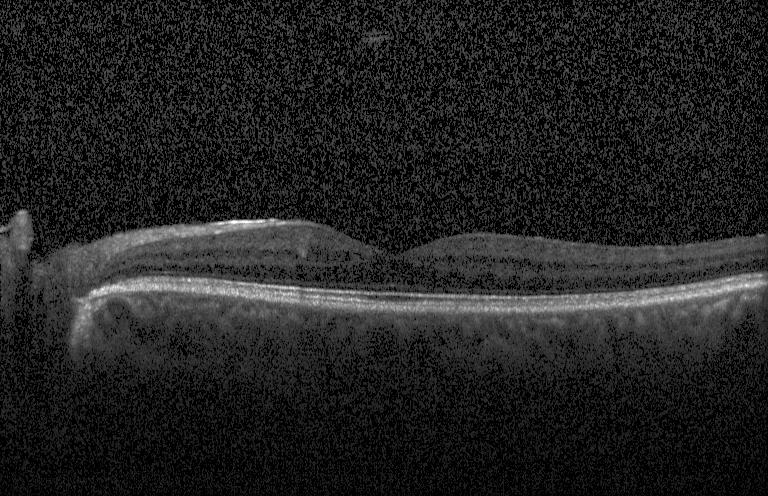
SD-OCT, fovea-centered, optical coherence tomography B-scan
Impression: neither choroidal neovascularization, diabetic macular edema, nor drusen.